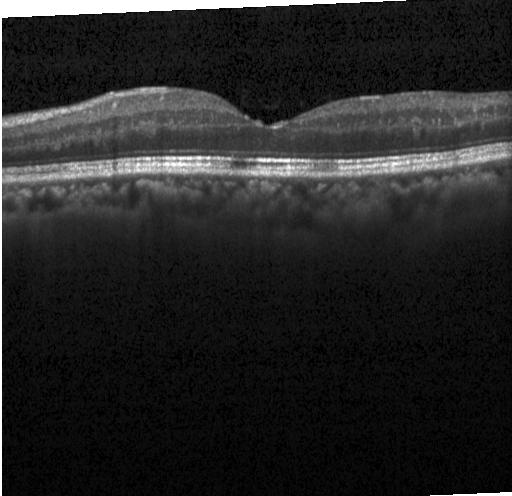
Impression: no choroidal neovascularization, diabetic macular edema, or drusen.